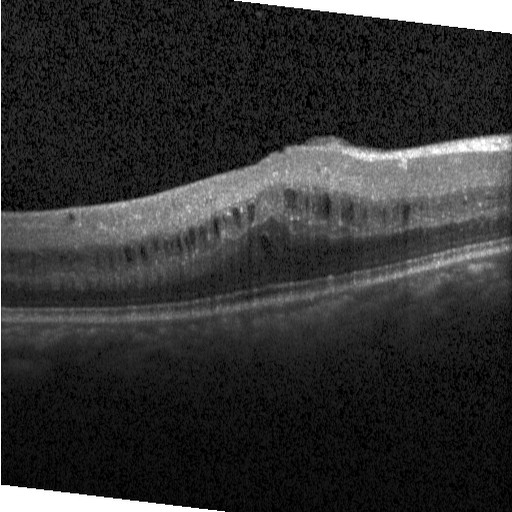 Heidelberg Spectralis OCT system. Retinal OCT B-scan. Spectral-domain optical coherence tomography. Horizontal scan through the fovea. Dx: DME.